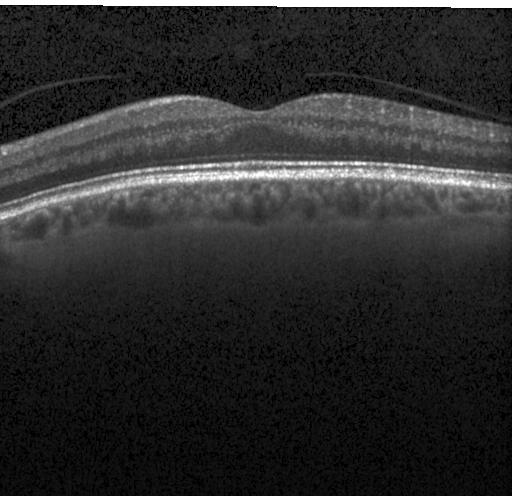

OCT line scan. No choroidal neovascularization, diabetic macular edema, or drusen.